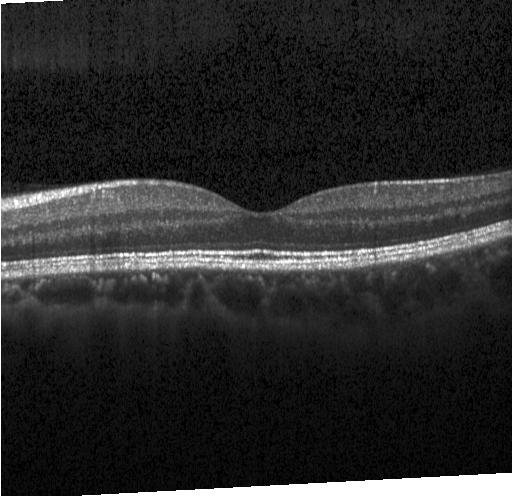
Spectral-domain OCT; through the macula; retinal OCT cross-section; Heidelberg Spectralis. Finding: neither choroidal neovascularization, diabetic macular edema, nor drusen.